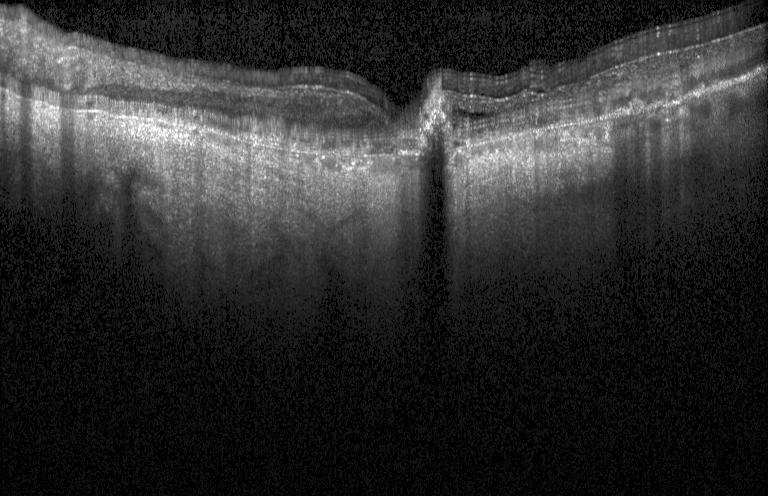

Heidelberg Spectralis OCT system, OCT B-scan, spectral-domain OCT, centered on the fovea. Assessment: CNV.